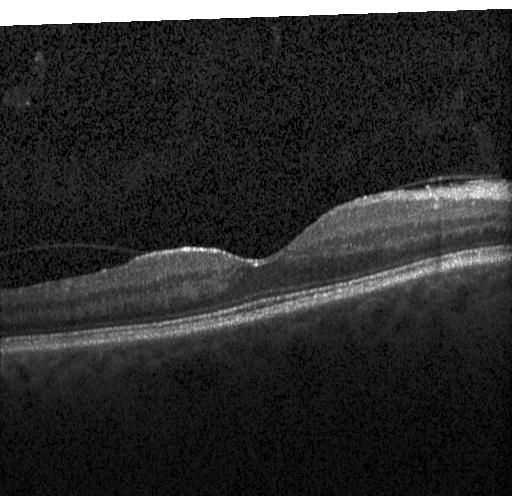

No choroidal neovascularization, diabetic macular edema, or drusen.